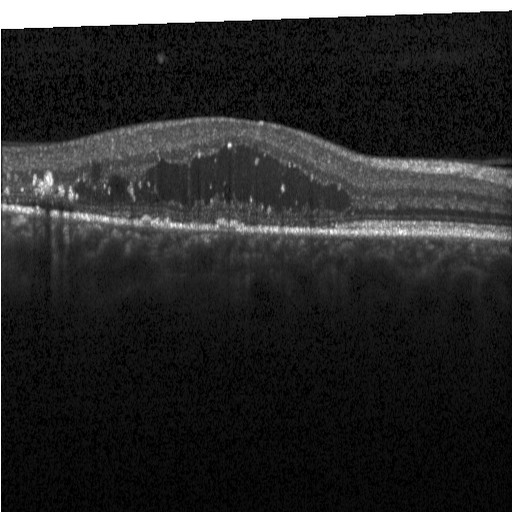
OCT B-scan. Spectral-domain optical coherence tomography. Heidelberg Spectralis OCT system.
This B-scan demonstrates diabetic macular edema.